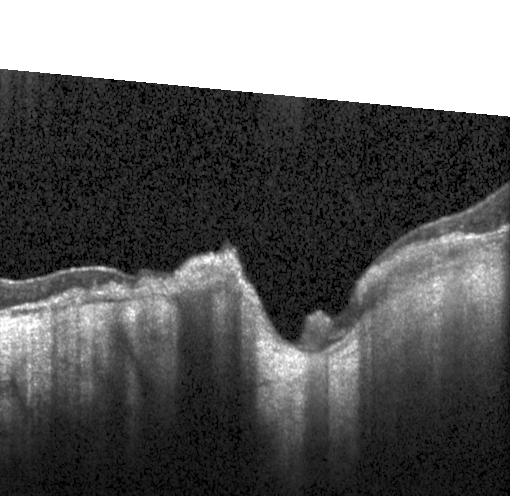
Horizontal scan through the fovea · optical coherence tomography scan
Finding: a choroidal neovascular membrane.